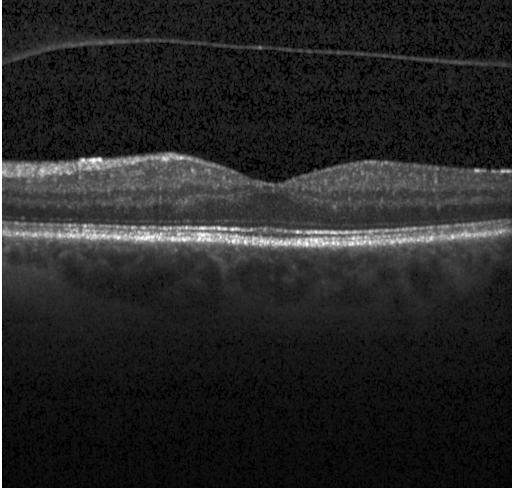 Macular OCT demonstrating neither choroidal neovascularization, diabetic macular edema, nor drusen.